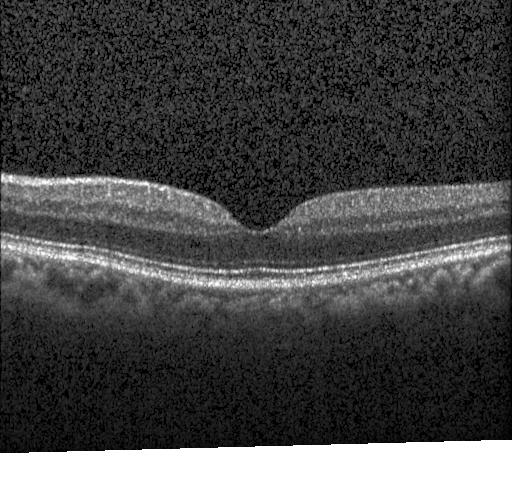 Spectral-domain optical coherence tomography; through the macula; acquired on a Heidelberg Spectralis; retinal OCT B-scan — This B-scan demonstrates neither CNV, DME, nor drusen.